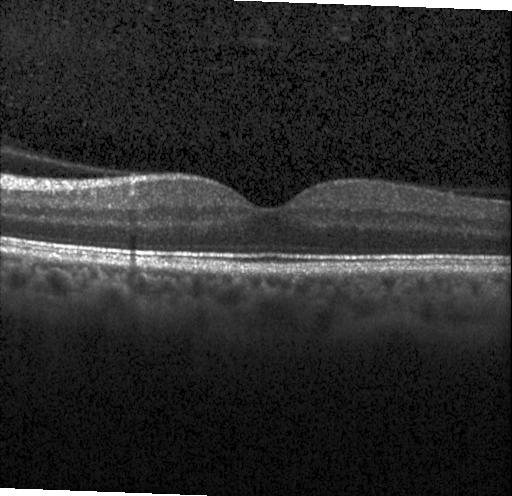 Centered on the fovea; optical coherence tomography B-scan; SD-OCT; instrument: Heidelberg Spectralis. Diagnosis: neither choroidal neovascularization, diabetic macular edema, nor drusen.